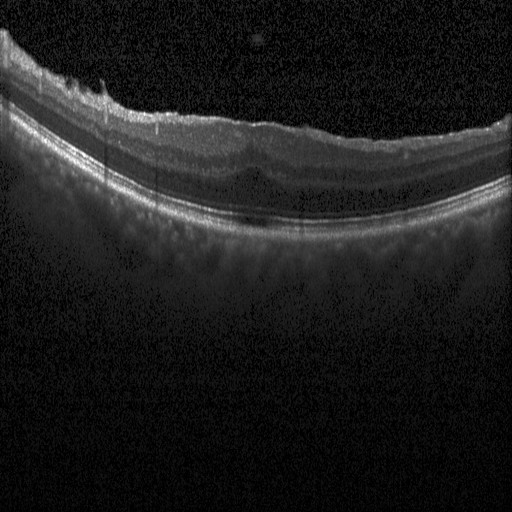

Retinal OCT B-scan · macular scan · SD-OCT · acquired on a Heidelberg Spectralis. Finding: diabetic macular edema (DME).